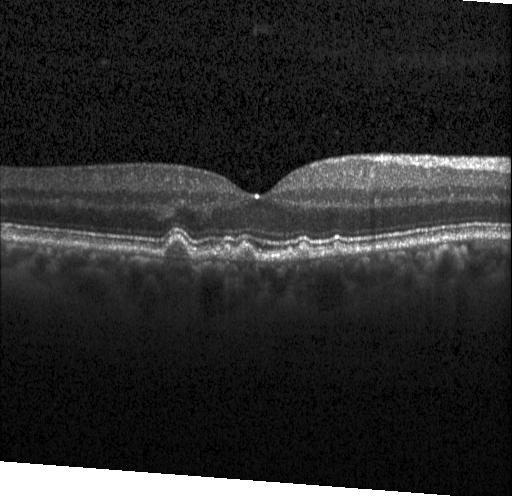
Finding: drusen.